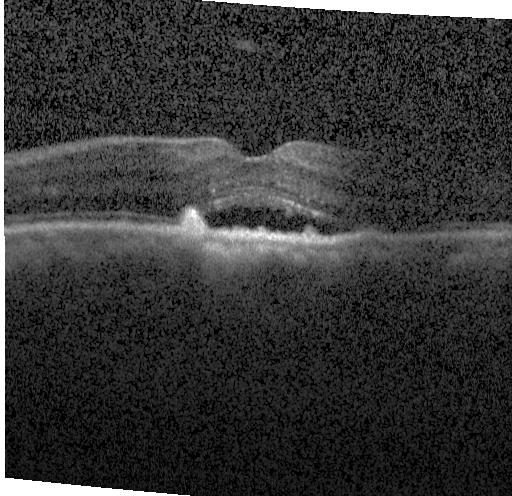 Spectral-domain optical coherence tomography · fovea-centered · OCT line scan — Assessment: choroidal neovascularization.